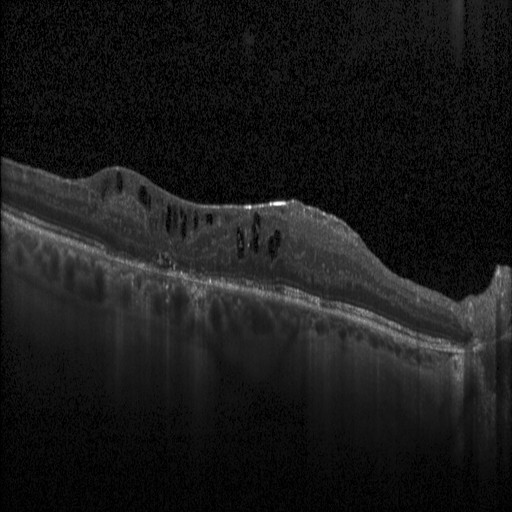

SD-OCT; retinal OCT cross-section. The scan shows DME.